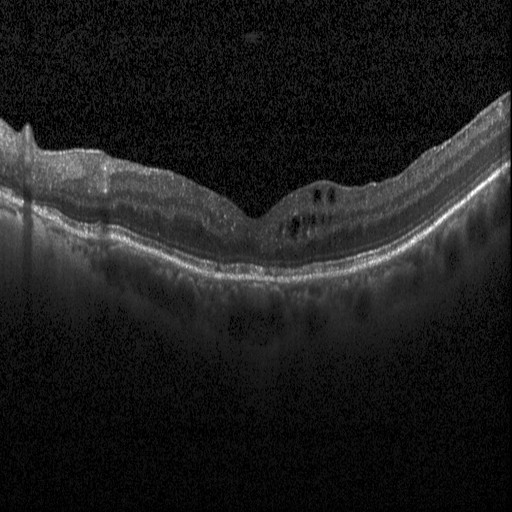
Centered on the fovea; retinal OCT B-scan. Dx: DME.